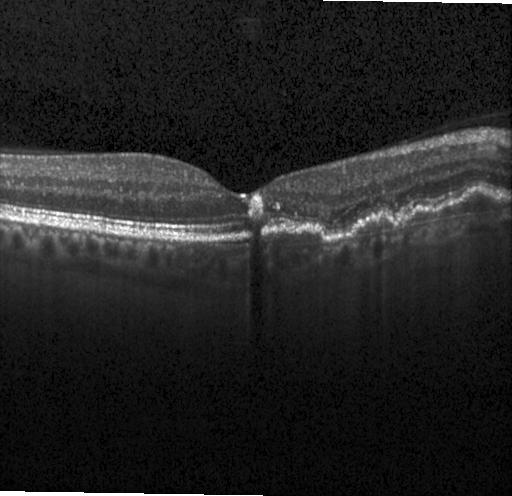 OCT line scan · acquired on a Heidelberg Spectralis · spectral-domain OCT. Dx: choroidal neovascularization (CNV).